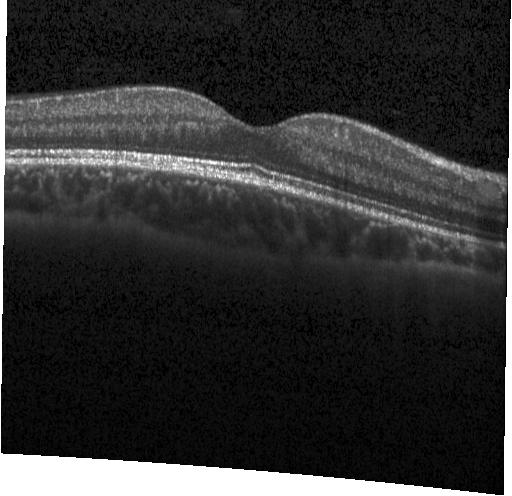

The scan shows no CNV, DME, or drusen.